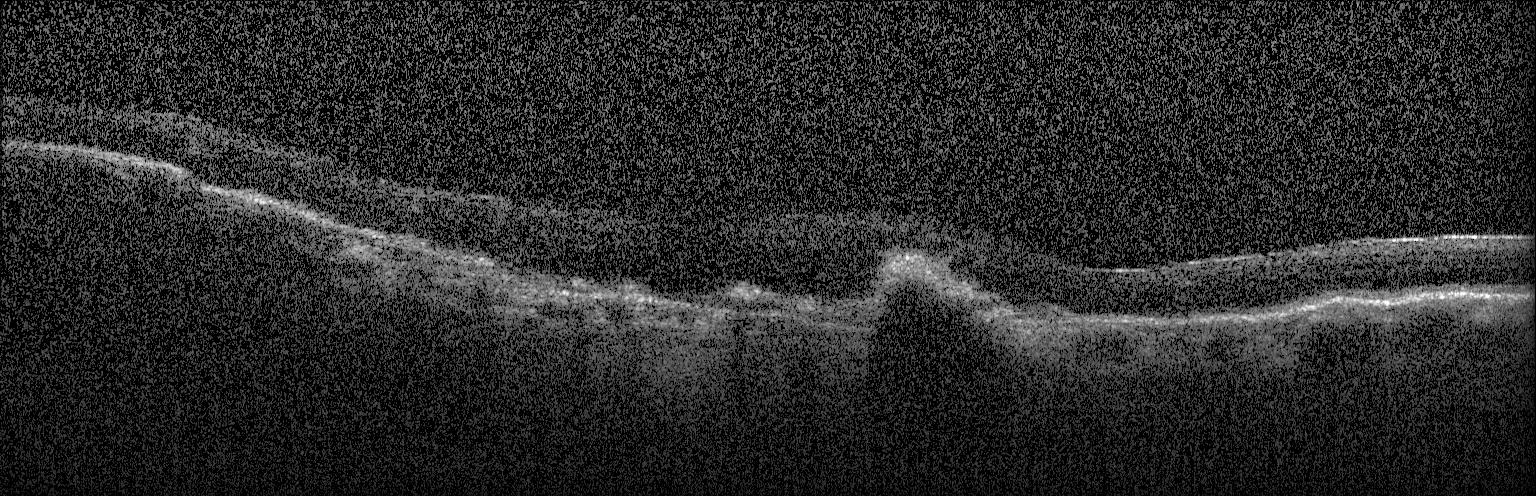

Centered on the fovea · retinal OCT B-scan · SD-OCT · acquired on a Heidelberg Spectralis
Diagnosis: choroidal neovascularization.